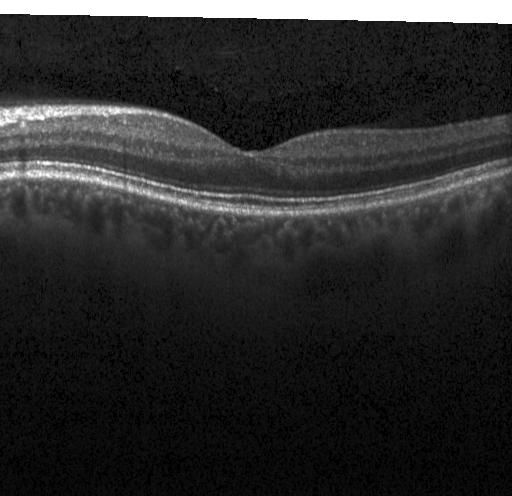

Fovea-centered, SD-OCT, OCT B-scan, Heidelberg Spectralis.
Dx: no evidence of CNV, DME, or drusen.